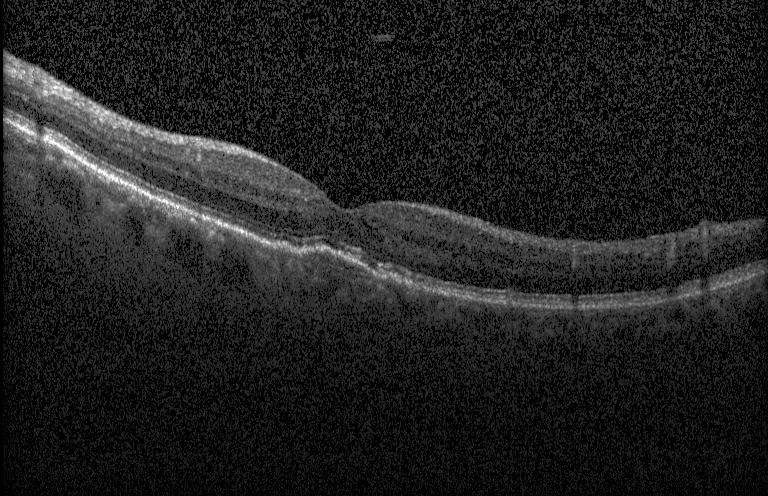 Optical coherence tomography B-scan · through the macula.
Macular OCT: a choroidal neovascular membrane.